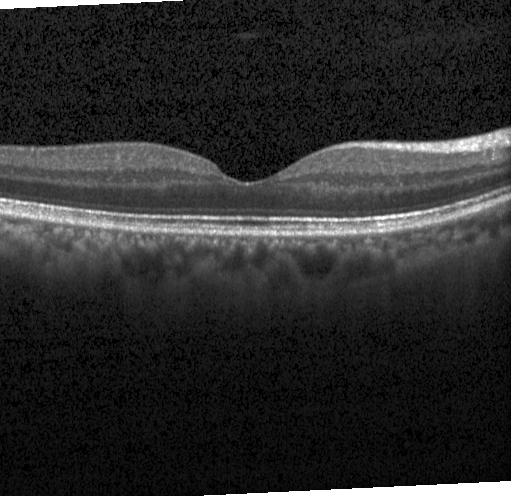 Optical coherence tomography B-scan.
Finding: no evidence of choroidal neovascularization, diabetic macular edema, or drusen.